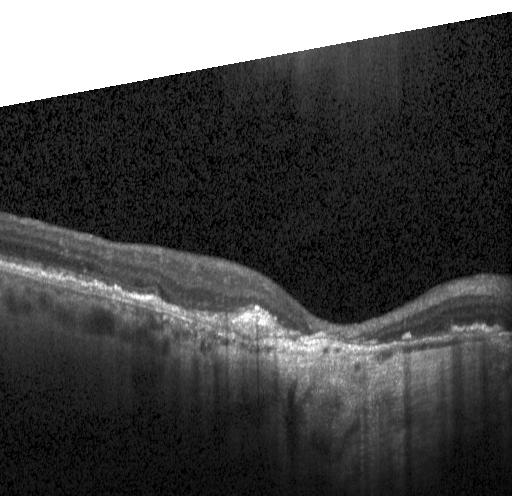

Through the macula, SD-OCT, OCT line scan. Finding: choroidal neovascularization (CNV).